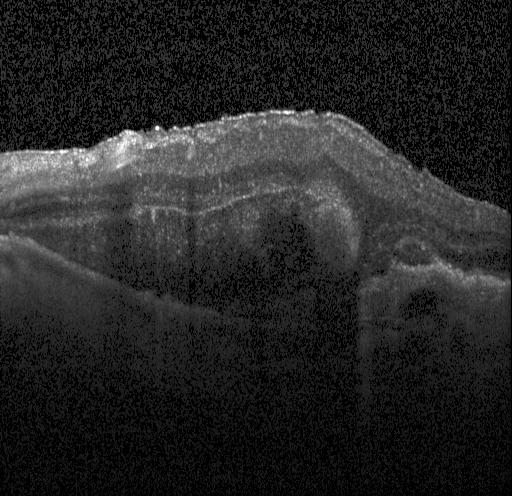

OCT B-scan · spectral-domain optical coherence tomography · fovea-centered · instrument: Heidelberg Spectralis.
Dx: choroidal neovascularization.